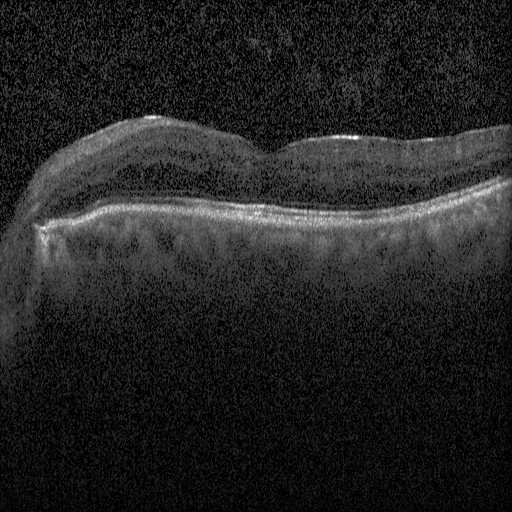

Optical coherence tomography B-scan; SD-OCT — Assessment: diabetic macular edema.